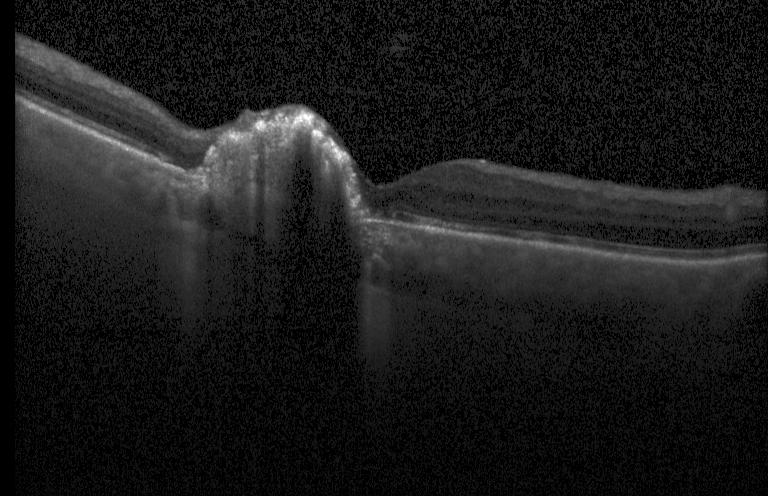 Retinal OCT cross-section. Heidelberg Spectralis OCT system. Macular scan — A choroidal neovascular membrane.